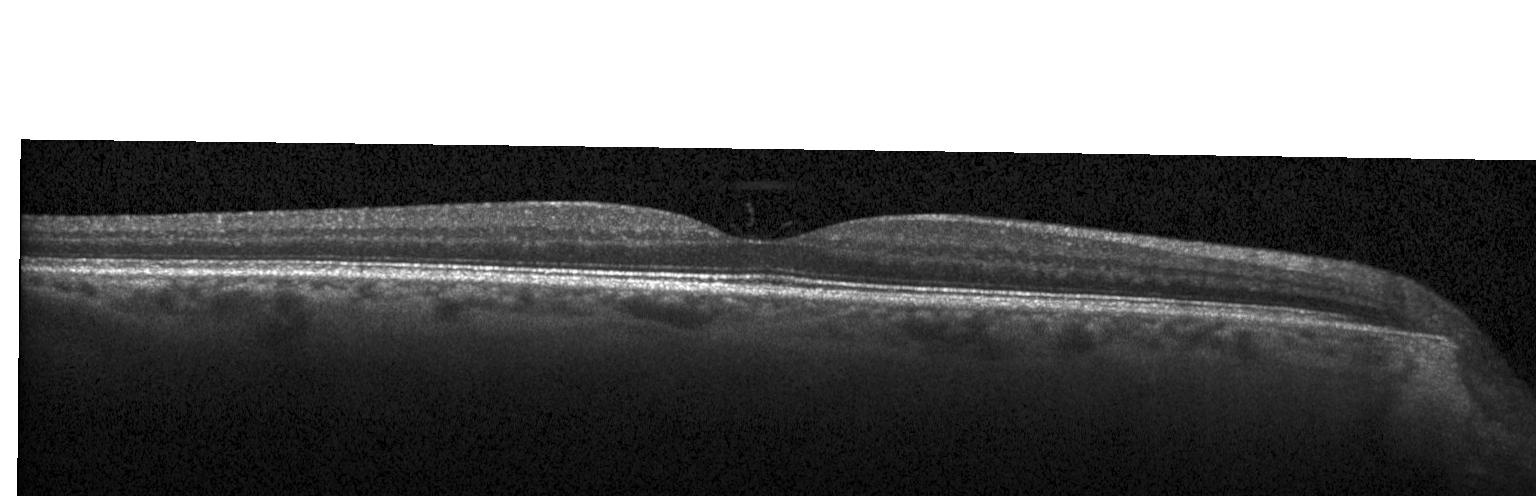

Macular OCT: neither choroidal neovascularization, diabetic macular edema, nor drusen.